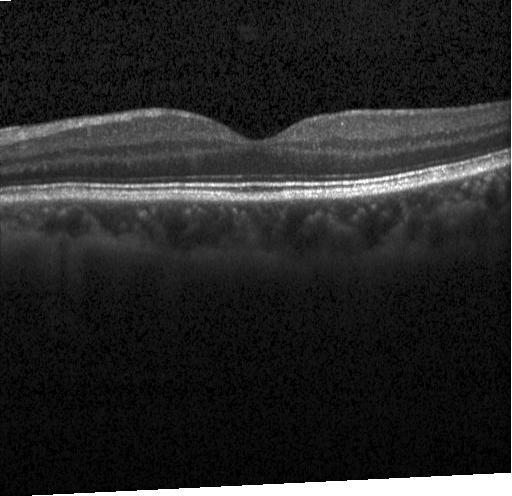

Horizontal scan through the fovea · spectral-domain optical coherence tomography · Heidelberg Spectralis · OCT line scan — No evidence of CNV, DME, or drusen.